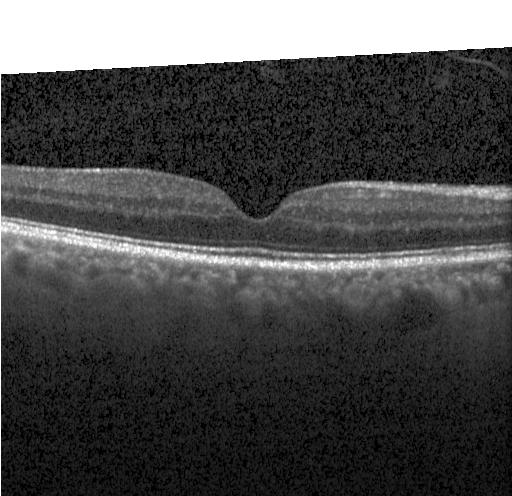 Centered on the fovea, instrument: Heidelberg Spectralis, SD-OCT, retinal OCT B-scan — Diagnosis: no choroidal neovascularization, diabetic macular edema, or drusen.